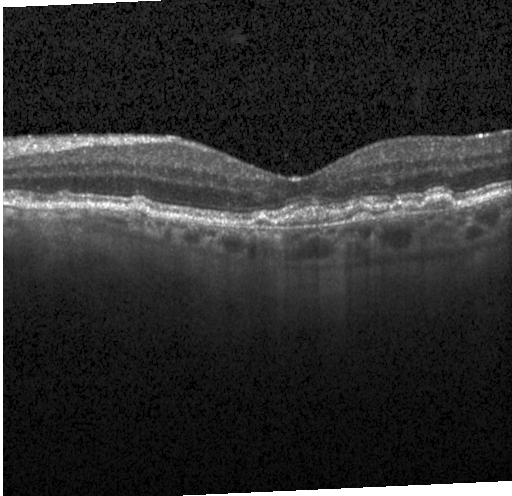

Centered on the fovea. Retinal OCT cross-section.
Diagnosis: a choroidal neovascular membrane.